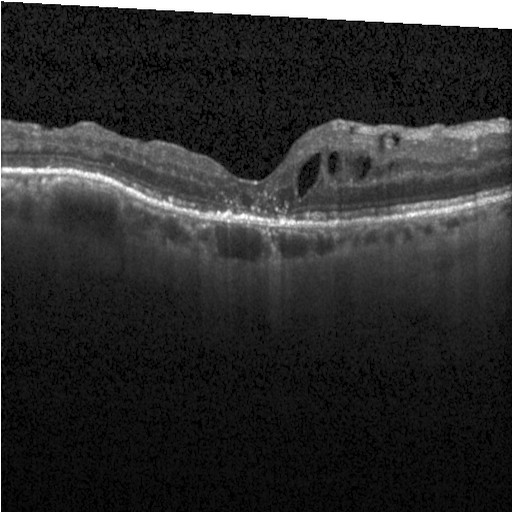

Retinal OCT cross-section · macular scan.
Assessment: diabetic macular edema (DME).